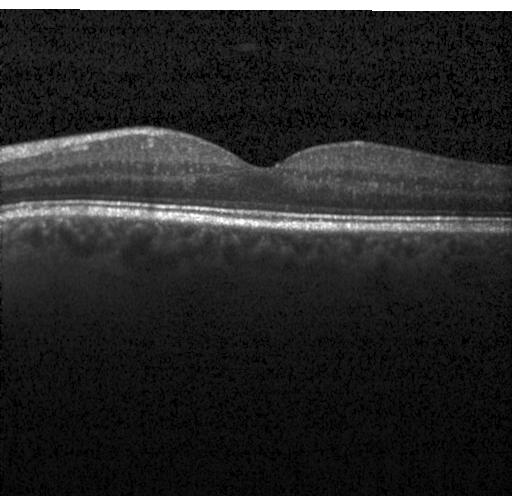 Horizontal scan through the fovea. OCT B-scan — Impression: no evidence of choroidal neovascularization, diabetic macular edema, or drusen.